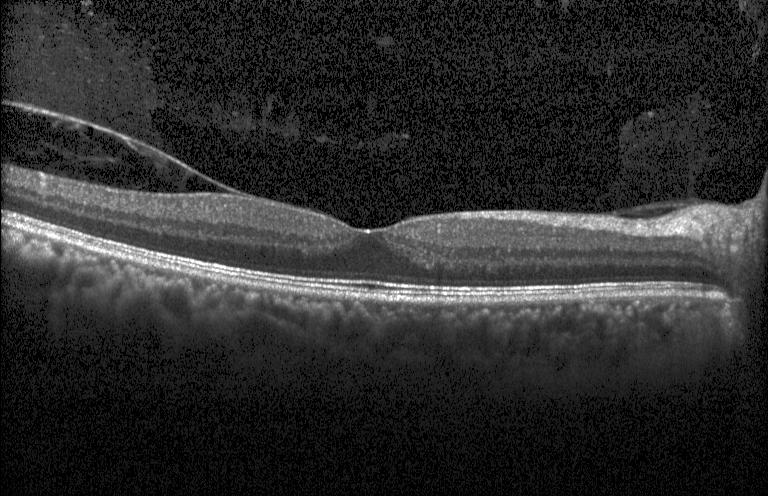
Finding: neither choroidal neovascularization, diabetic macular edema, nor drusen.